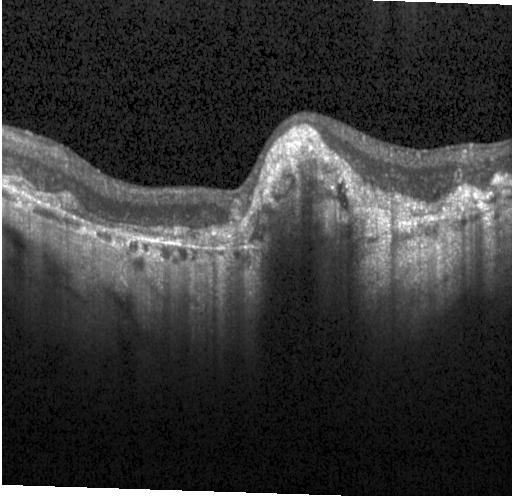

Macular OCT: a choroidal neovascular membrane.